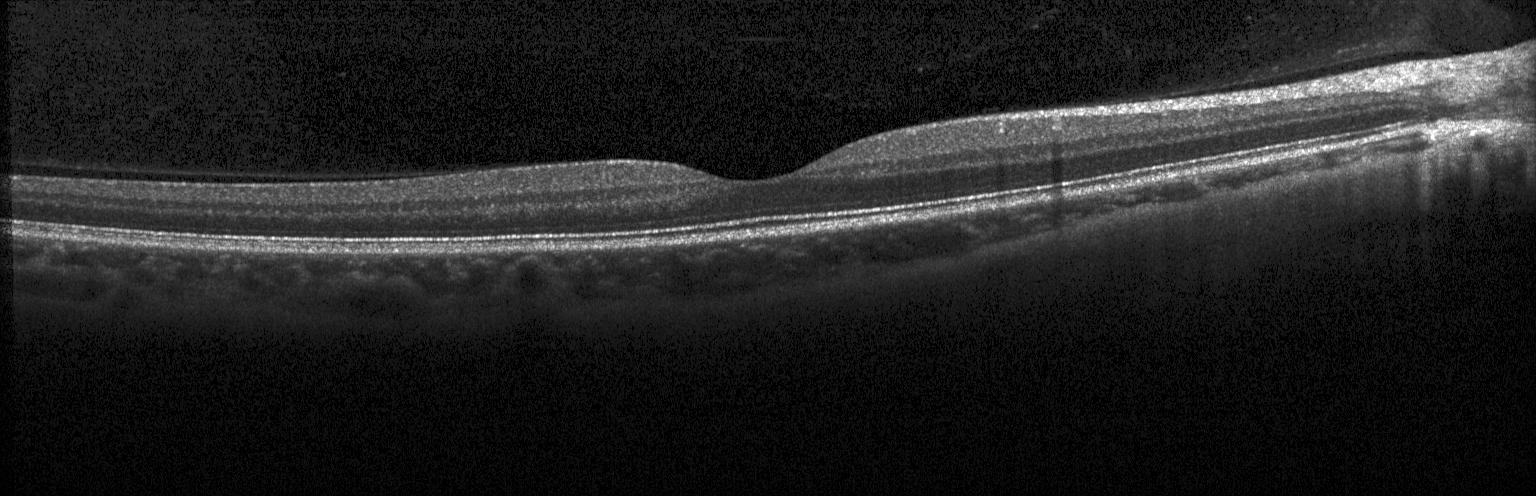 Acquired on a Heidelberg Spectralis; OCT B-scan; spectral-domain optical coherence tomography; fovea-centered.
Dx: no choroidal neovascularization, no diabetic macular edema, and no drusen.